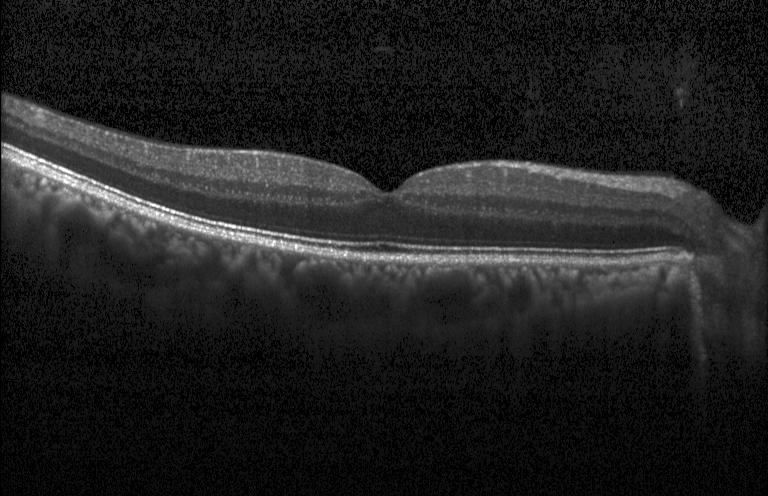
OCT B-scan, centered on the fovea, SD-OCT.
Assessment: no choroidal neovascularization, no diabetic macular edema, and no drusen.